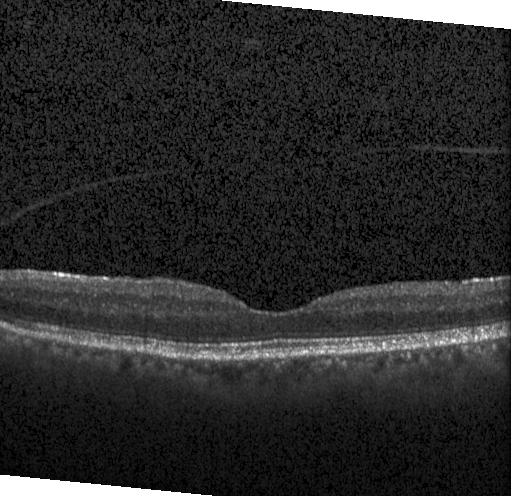 Macular OCT demonstrating no evidence of choroidal neovascularization, diabetic macular edema, or drusen.